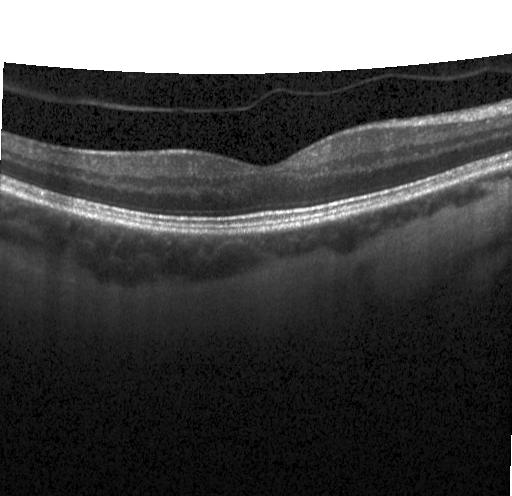

Spectral-domain OCT. Acquired on a Heidelberg Spectralis. Retinal OCT cross-section — Impression: no choroidal neovascularization, diabetic macular edema, or drusen.